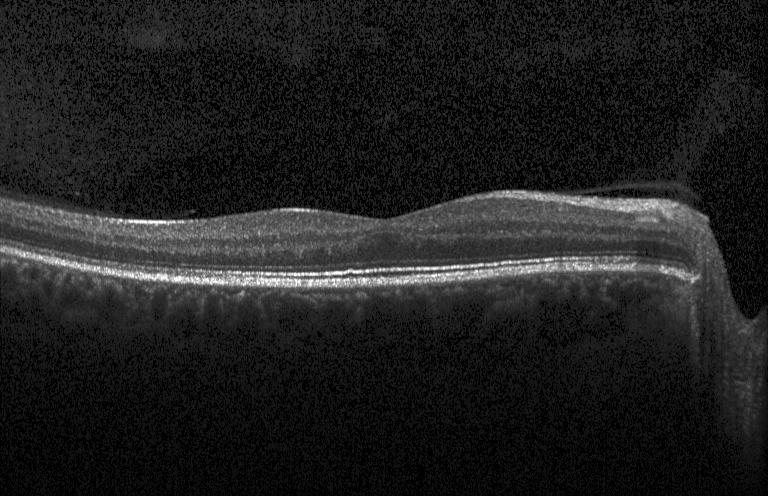

This B-scan demonstrates no choroidal neovascularization, diabetic macular edema, or drusen.